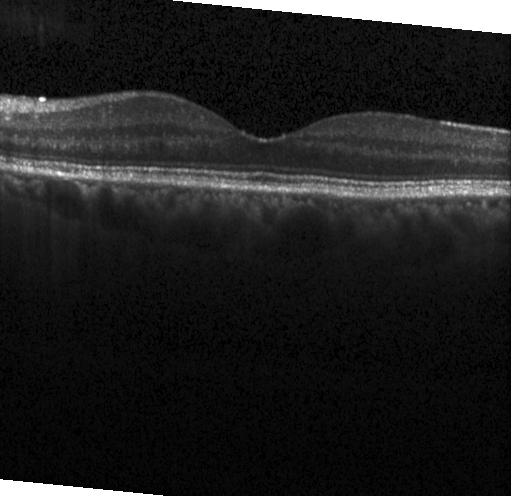
Spectral-domain optical coherence tomography. Retinal OCT cross-section. Instrument: Heidelberg Spectralis
Finding: neither choroidal neovascularization, diabetic macular edema, nor drusen.